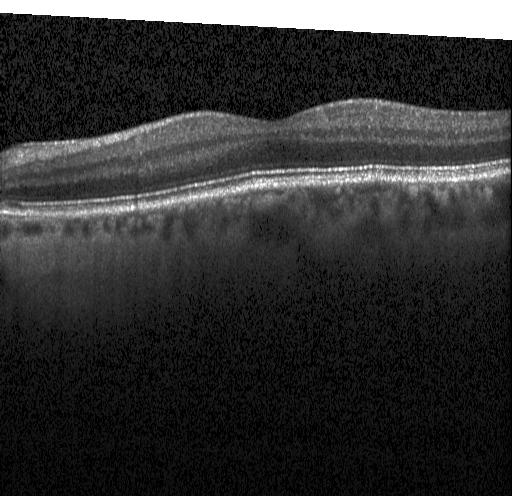
Optical coherence tomography B-scan.
Impression: neither choroidal neovascularization, diabetic macular edema, nor drusen.